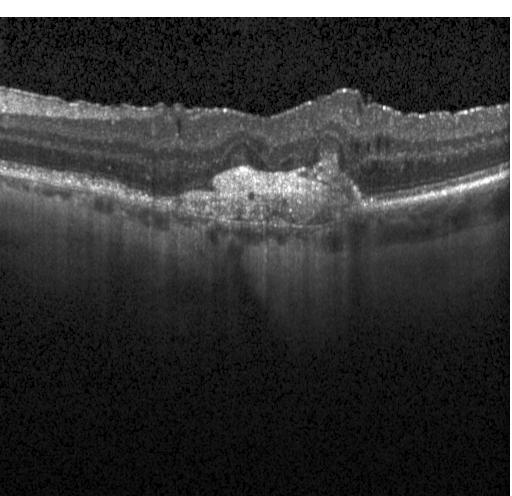
Optical coherence tomography B-scan.
The scan shows a choroidal neovascular membrane.